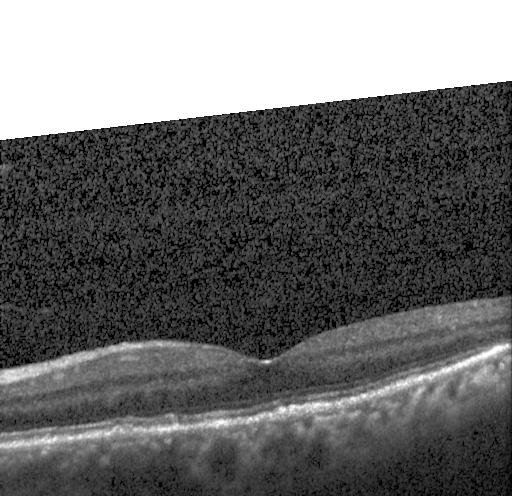 OCT line scan — Assessment: drusen.